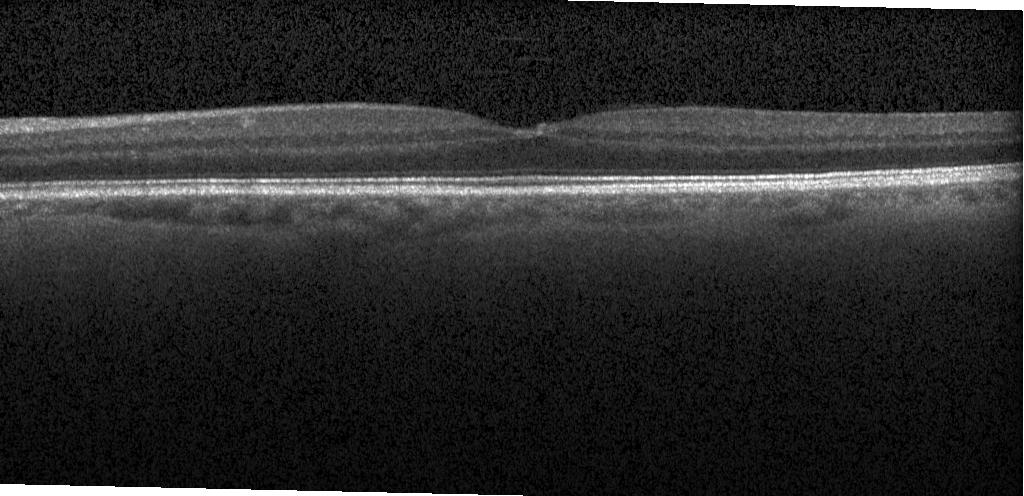

Diagnosis: no evidence of choroidal neovascularization, diabetic macular edema, or drusen.